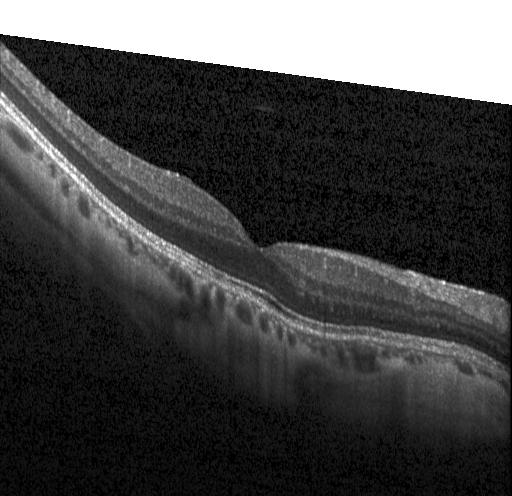

Macular scan. Spectral-domain optical coherence tomography. Retinal OCT B-scan. Acquired on a Heidelberg Spectralis
Assessment: no evidence of CNV, DME, or drusen.